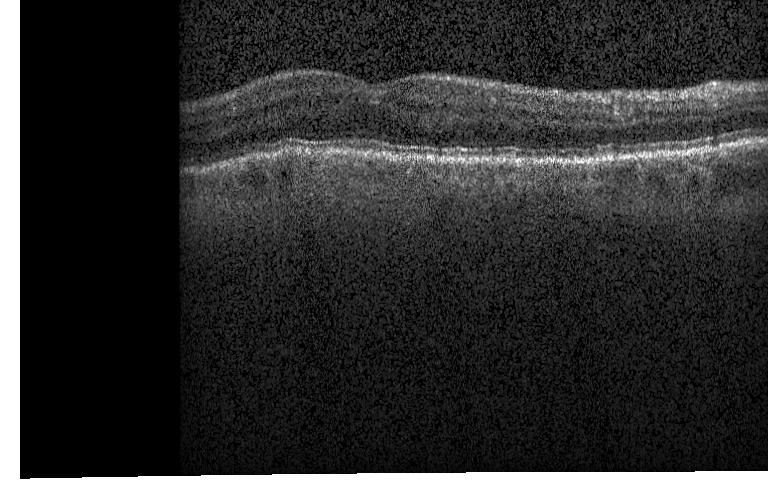 SD-OCT. Optical coherence tomography B-scan. Heidelberg Spectralis OCT system. Centered on the fovea.
Dx: no evidence of choroidal neovascularization, diabetic macular edema, or drusen.